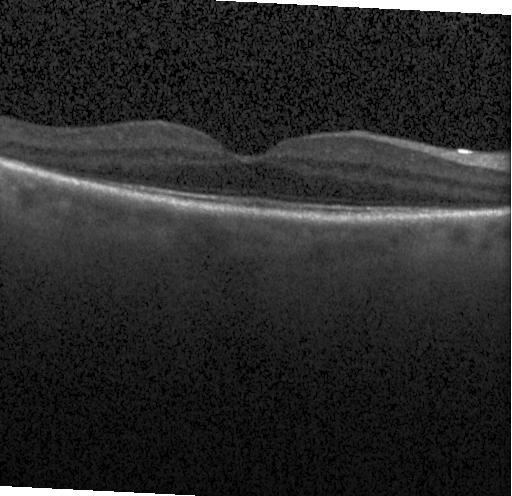
Retinal OCT B-scan.
OCT finding: neither choroidal neovascularization, diabetic macular edema, nor drusen.